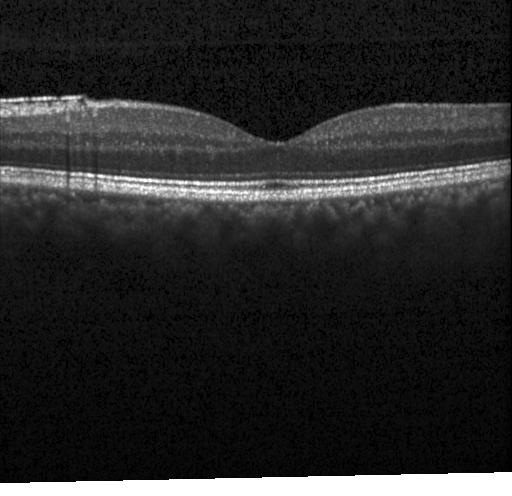 Spectral-domain OCT B-scan: no evidence of choroidal neovascularization, diabetic macular edema, or drusen.